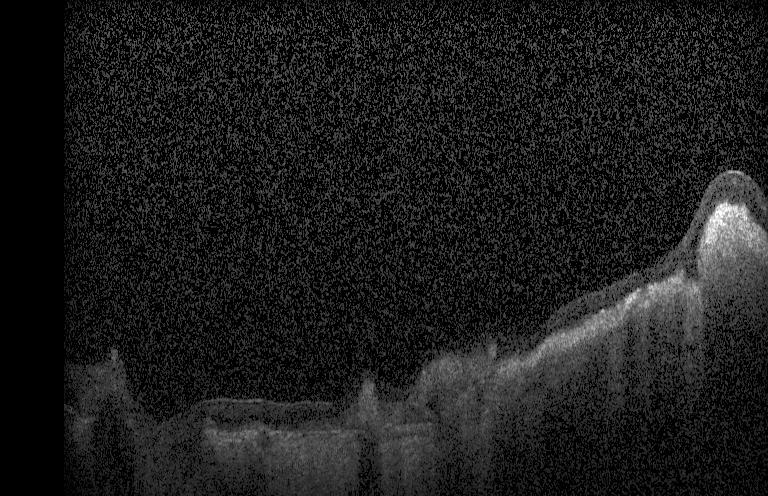
Retinal OCT B-scan · SD-OCT — Finding: CNV.